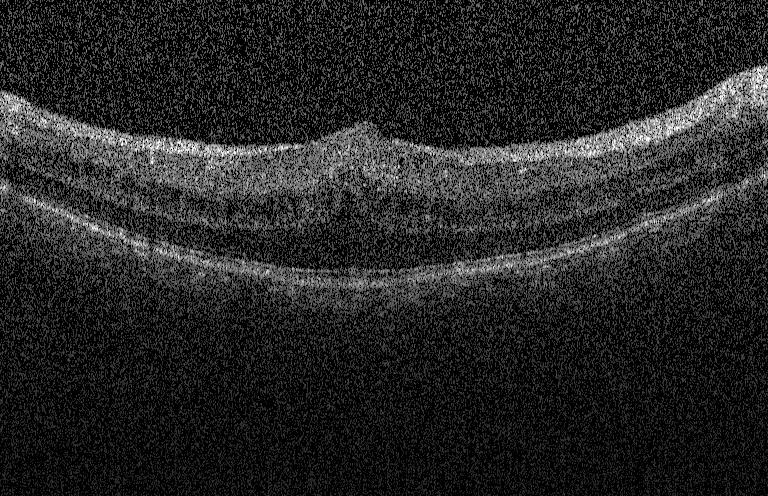

OCT scan showing diabetic macular edema.